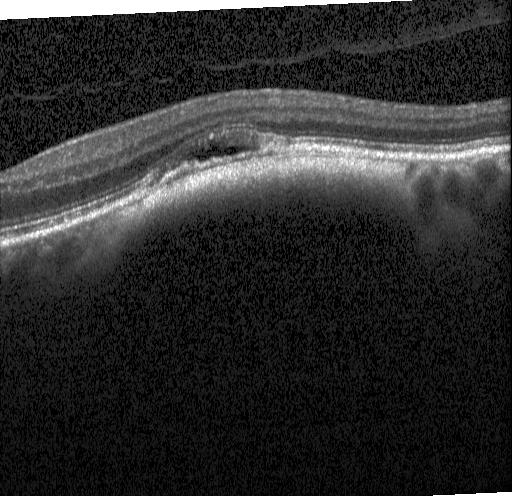

OCT B-scan. Fovea-centered. SD-OCT.
OCT finding: a choroidal neovascular membrane.